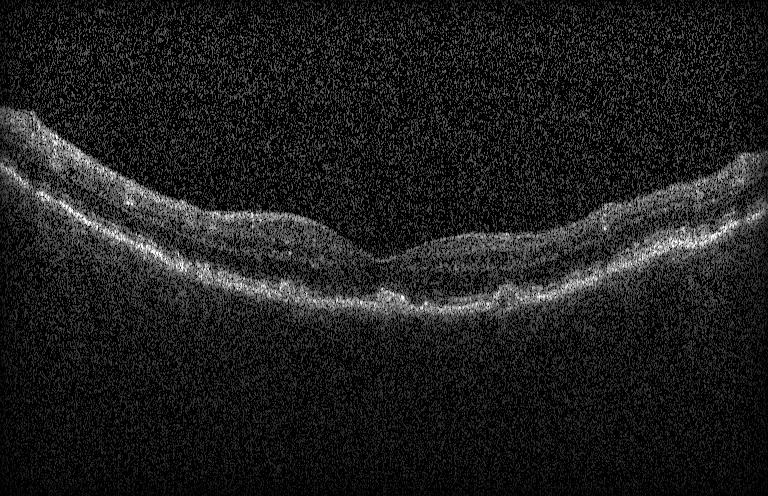

OCT finding: a choroidal neovascular membrane.